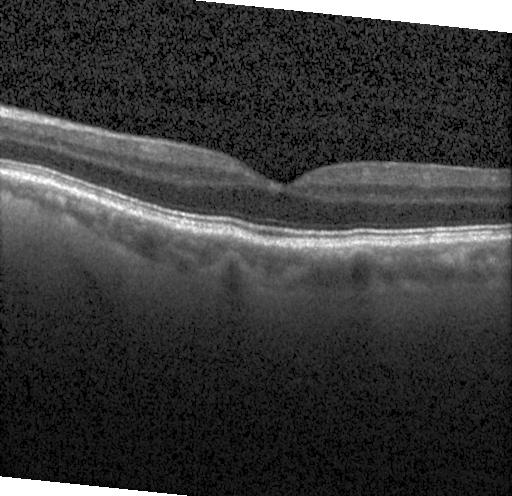
Dx: no evidence of choroidal neovascularization, diabetic macular edema, or drusen.